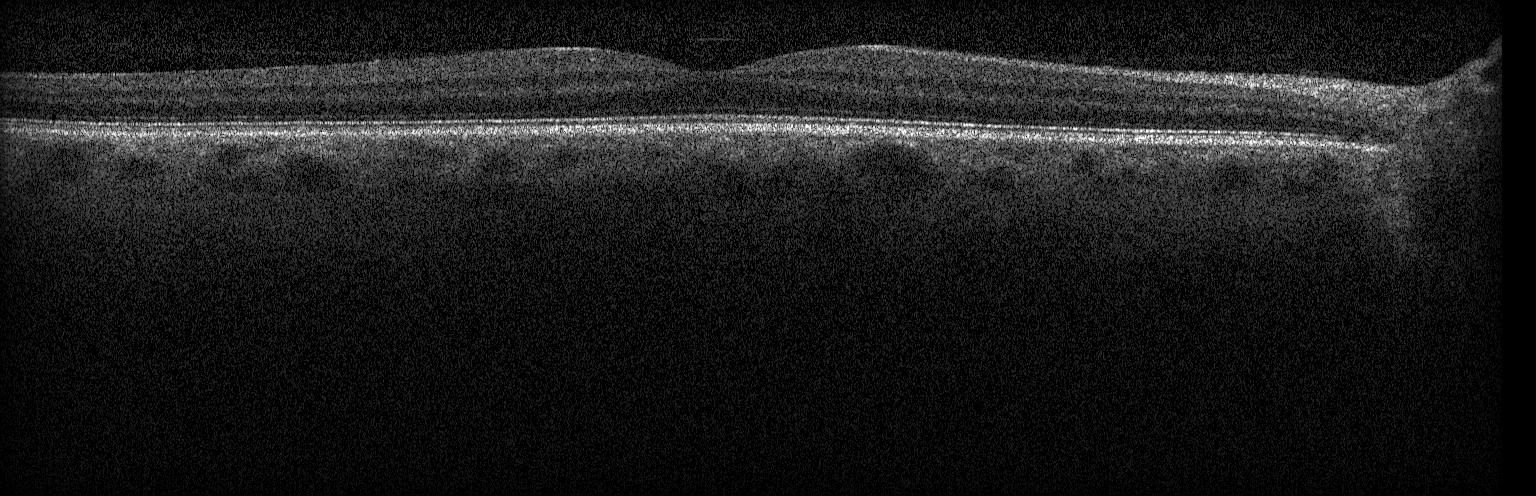

Spectral-domain OCT B-scan: neither choroidal neovascularization, diabetic macular edema, nor drusen.